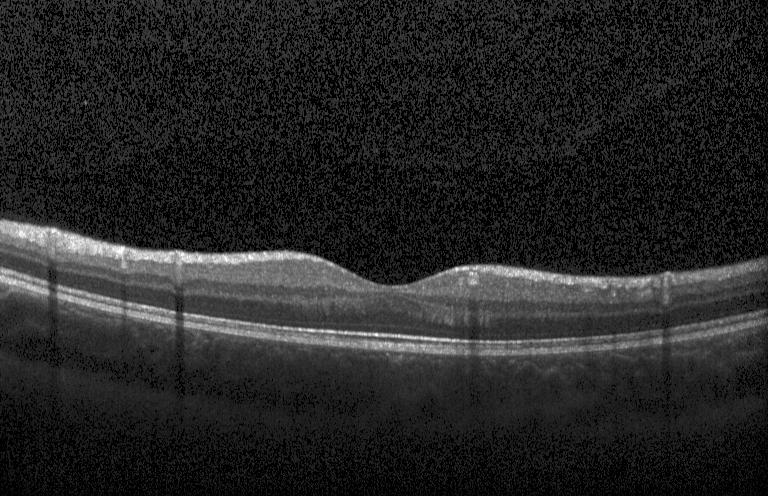 Instrument: Heidelberg Spectralis. OCT B-scan. This B-scan demonstrates no evidence of choroidal neovascularization, diabetic macular edema, or drusen.